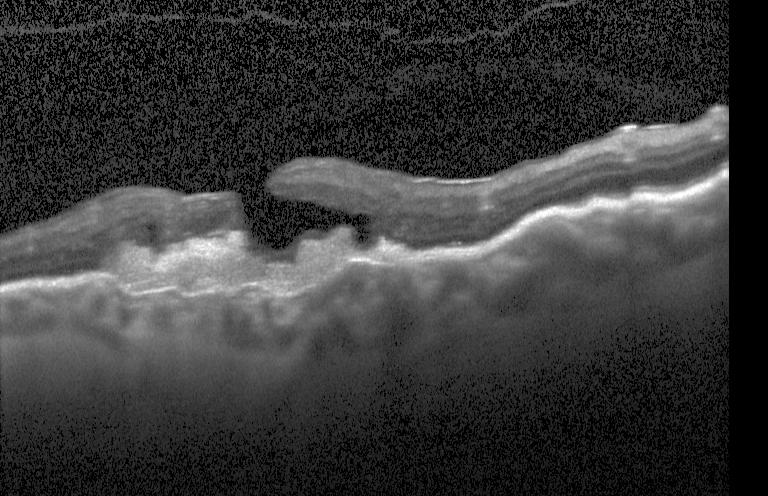

Macular scan · optical coherence tomography B-scan. Impression: choroidal neovascularization.